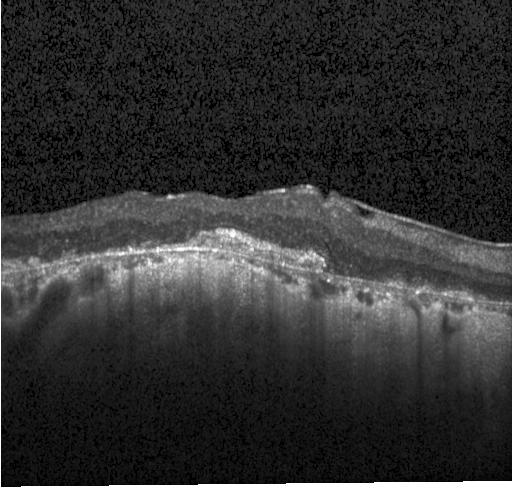 Impression: a choroidal neovascular membrane.